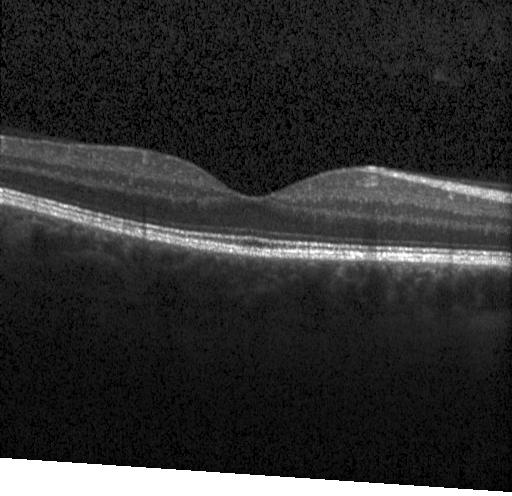 Fovea-centered · OCT line scan · spectral-domain optical coherence tomography · Heidelberg Spectralis — Assessment: neither choroidal neovascularization, diabetic macular edema, nor drusen.